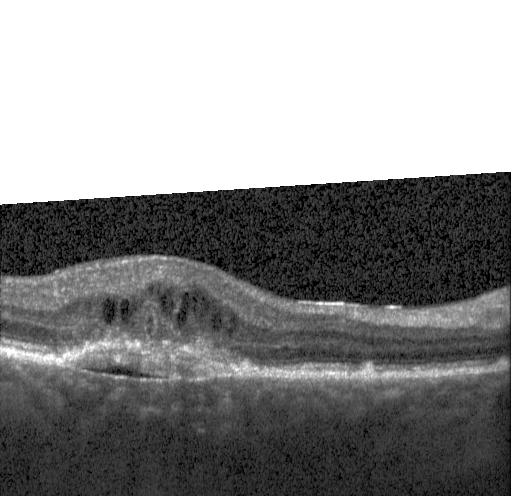
Optical coherence tomography B-scan — Assessment: a choroidal neovascular membrane.